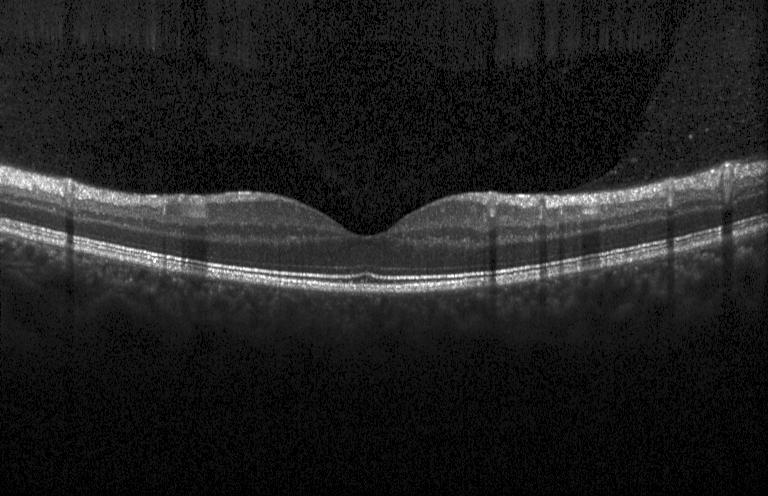
Retinal OCT cross-section. OCT finding: no evidence of CNV, DME, or drusen.